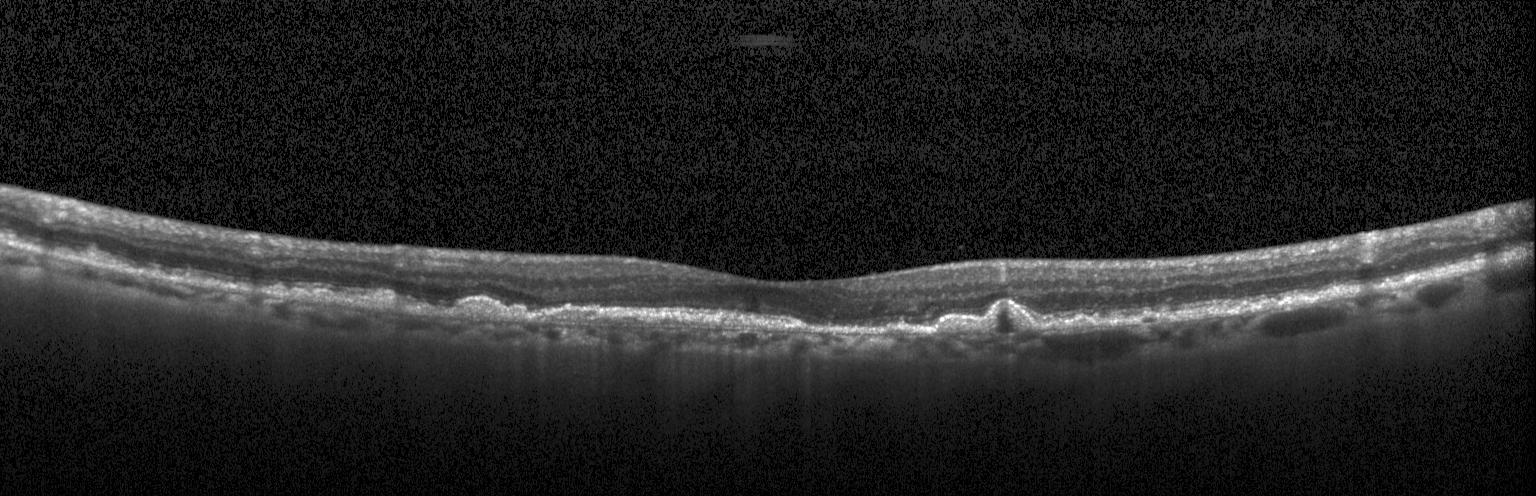

Retinal OCT cross-section; Heidelberg Spectralis; fovea-centered
Diagnosis: a choroidal neovascular membrane.